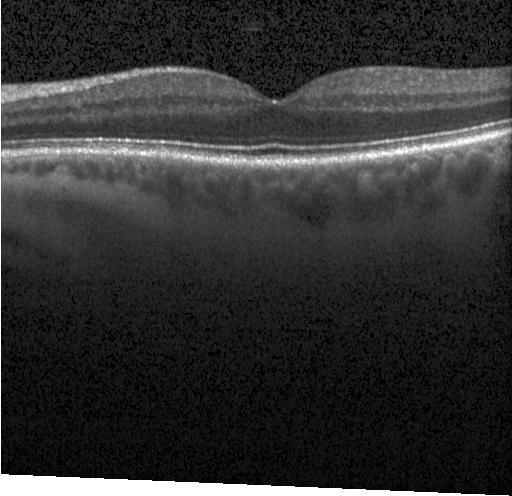
OCT B-scan — OCT finding: no choroidal neovascularization, diabetic macular edema, or drusen.